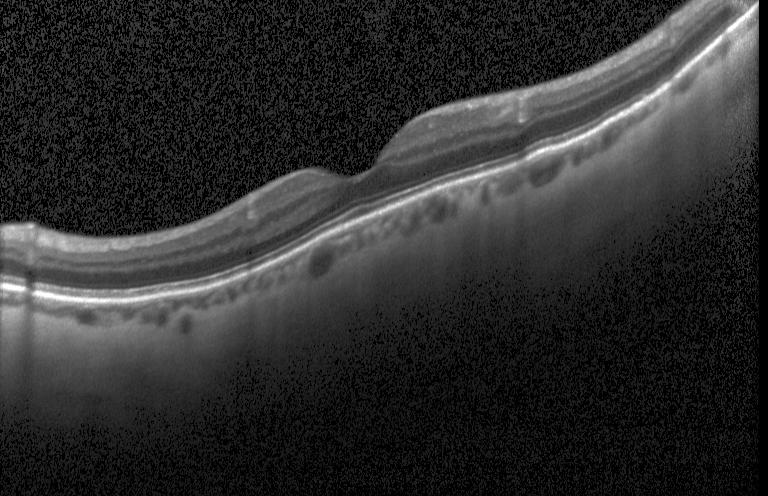 Optical coherence tomography scan. Spectral-domain optical coherence tomography.
Diagnosis: neither choroidal neovascularization, diabetic macular edema, nor drusen.